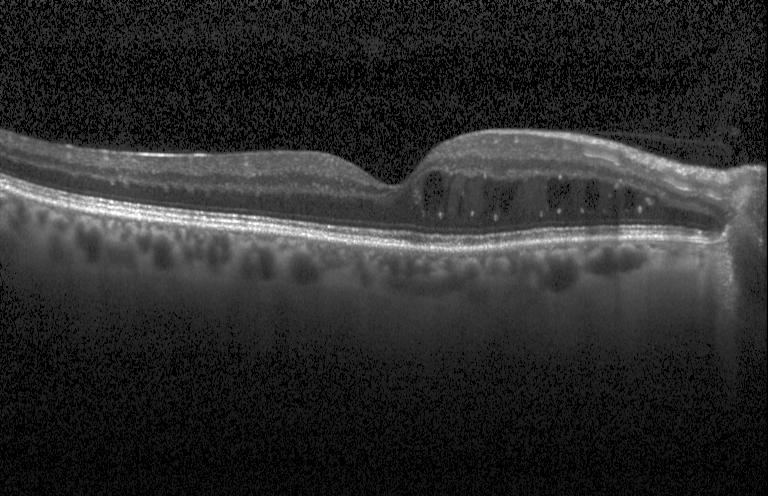
Heidelberg Spectralis; retinal OCT cross-section
The scan shows diabetic macular edema.